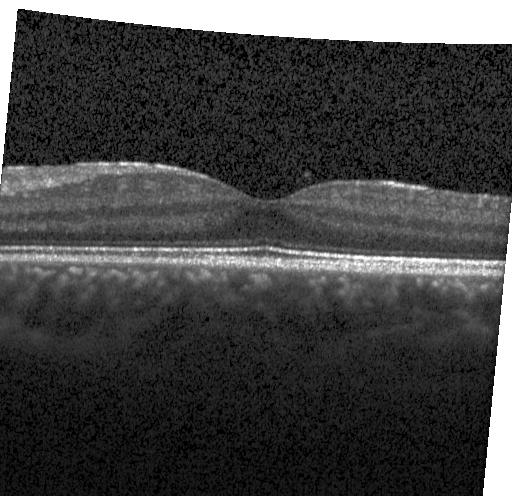 Diagnosis: no choroidal neovascularization, no diabetic macular edema, and no drusen.